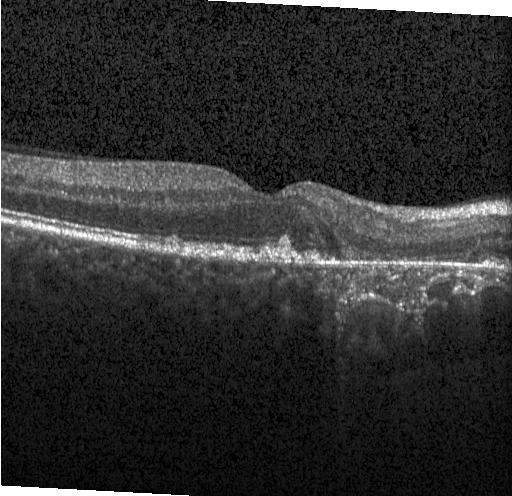

Macular OCT demonstrating CNV.